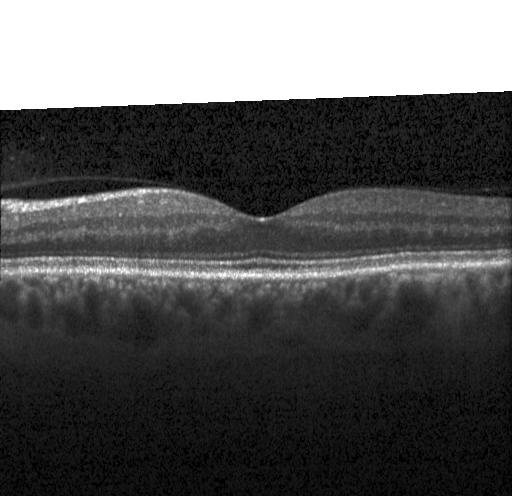

Optical coherence tomography B-scan.
Impression: no choroidal neovascularization, no diabetic macular edema, and no drusen.